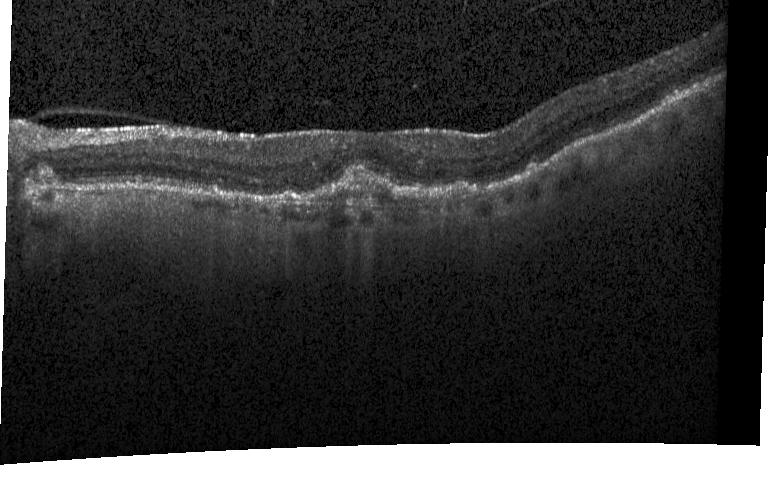 Heidelberg Spectralis; spectral-domain OCT; OCT B-scan; macular scan
Macular OCT: a choroidal neovascular membrane.